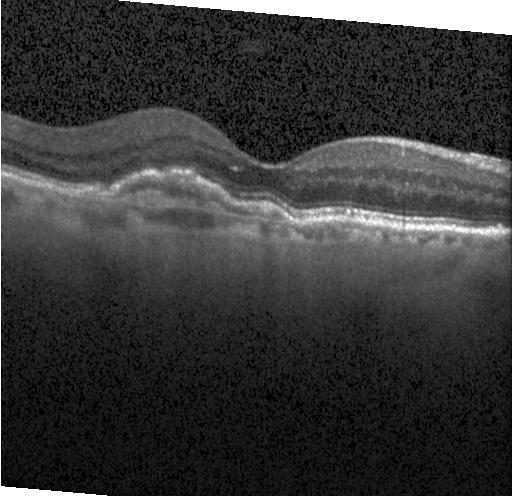

OCT B-scan. Fovea-centered.
The scan shows choroidal neovascularization (CNV).